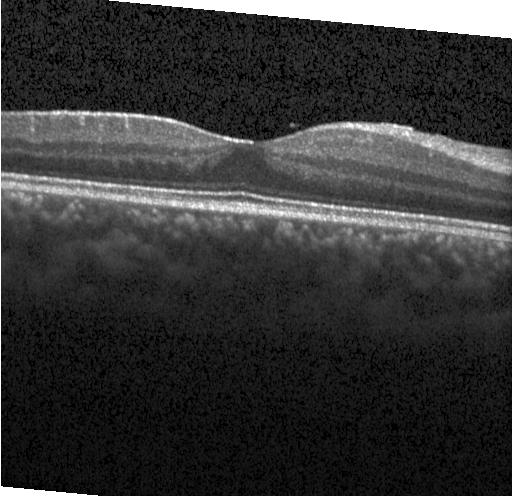
Macular scan · Heidelberg Spectralis · OCT B-scan — No evidence of CNV, DME, or drusen.